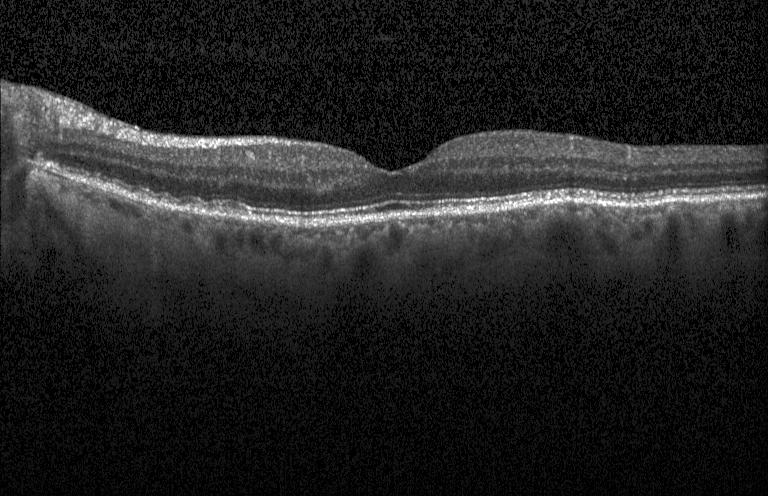 Macular OCT: drusen.